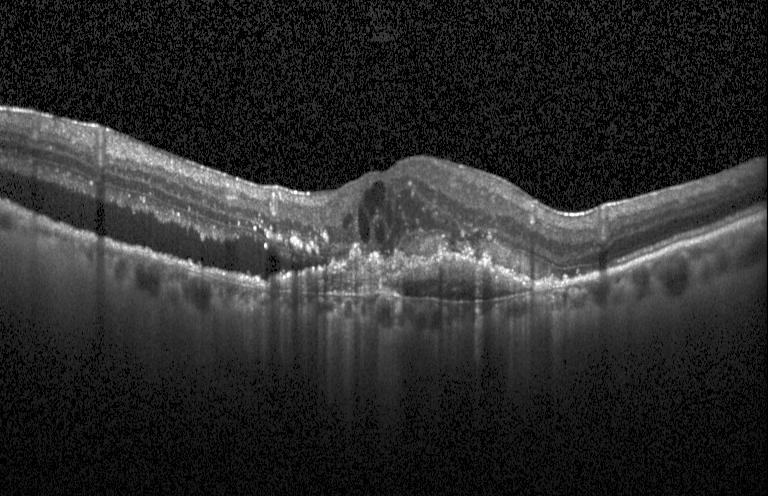 Optical coherence tomography scan; Heidelberg Spectralis OCT system; fovea-centered; spectral-domain optical coherence tomography — Diagnosis: choroidal neovascularization.